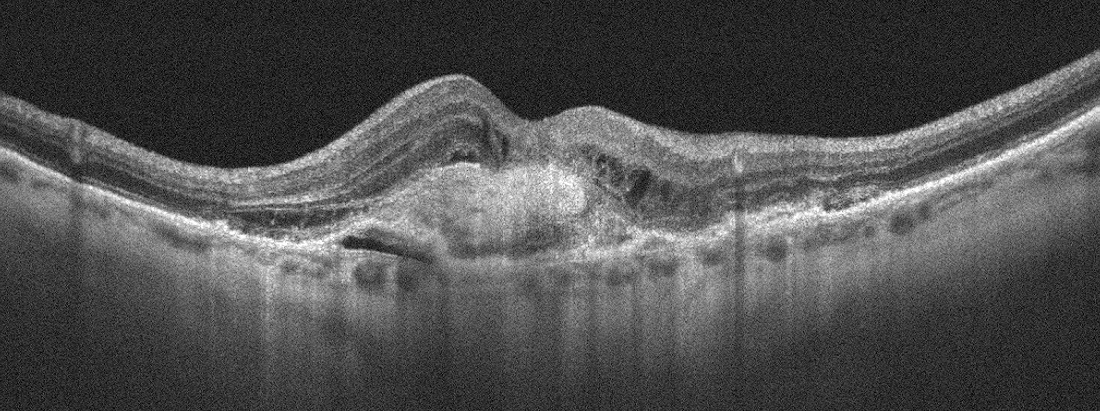

OCT B-scan showing age-related macular degeneration (AMD).